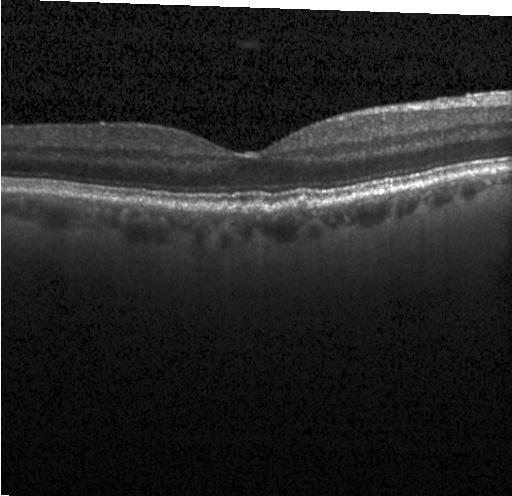

Instrument: Heidelberg Spectralis. Centered on the fovea. Optical coherence tomography scan. SD-OCT — Sub-RPE drusenoid deposits.